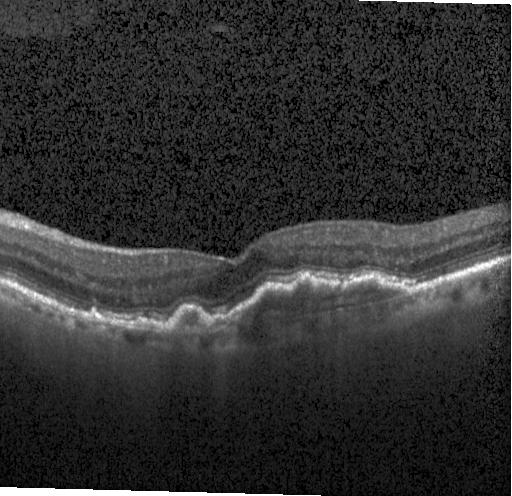
Centered on the fovea; spectral-domain optical coherence tomography; OCT line scan. Assessment: choroidal neovascularization.